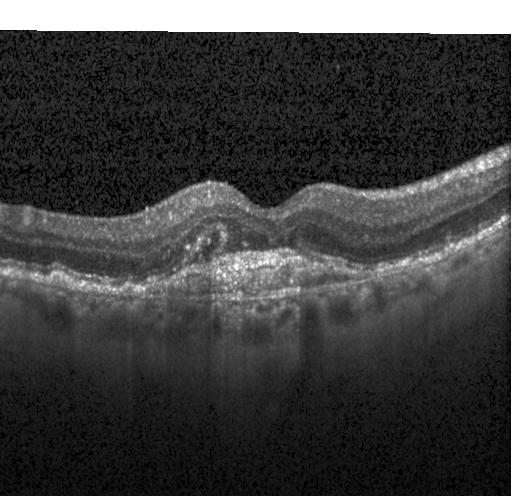 OCT B-scan; Heidelberg Spectralis; spectral-domain OCT; macular scan.
Assessment: choroidal neovascularization (CNV).